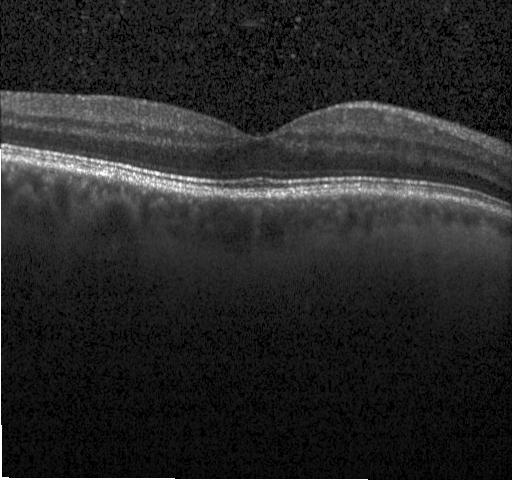 Macular OCT demonstrating no evidence of CNV, DME, or drusen.